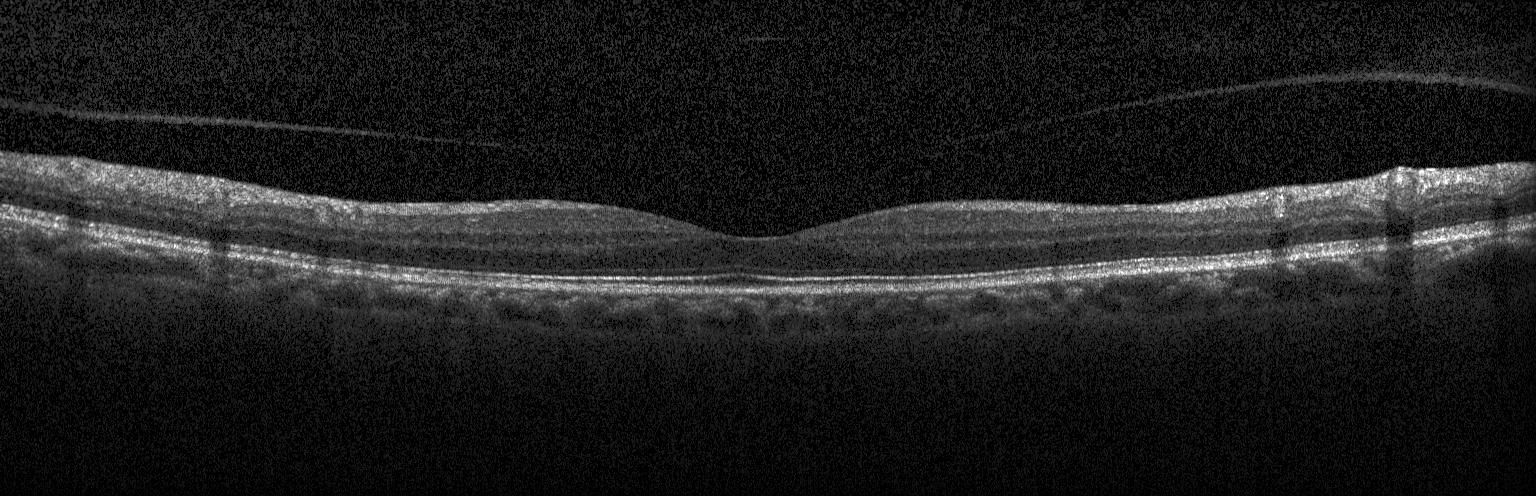

The scan shows no choroidal neovascularization, diabetic macular edema, or drusen.